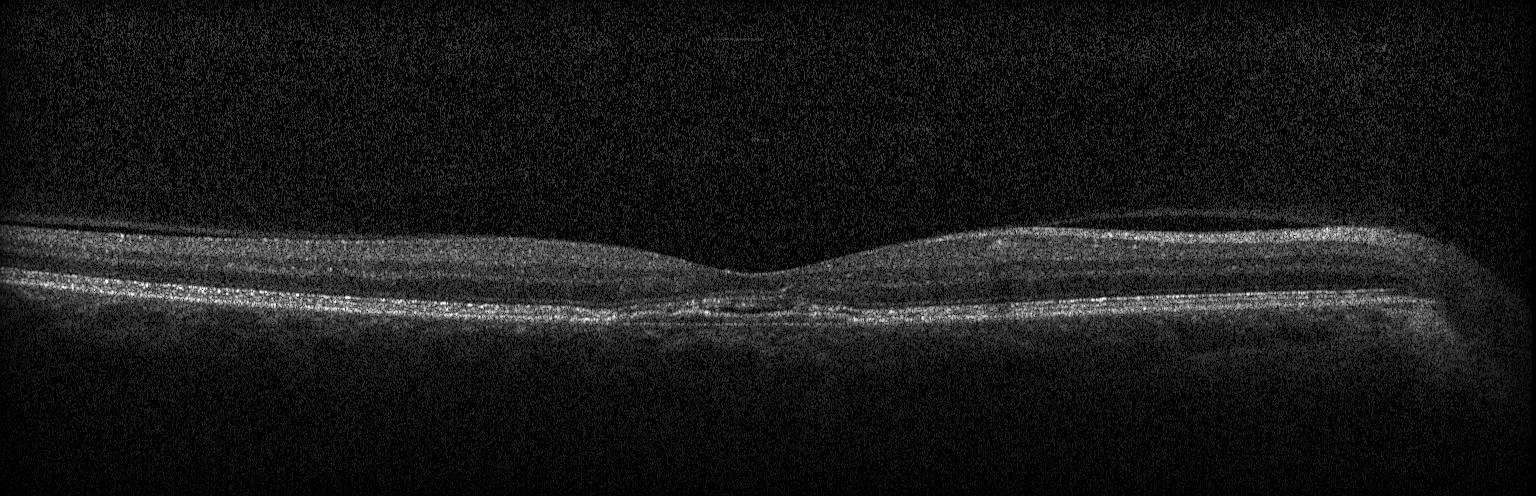
Optical coherence tomography scan, centered on the fovea.
CNV.